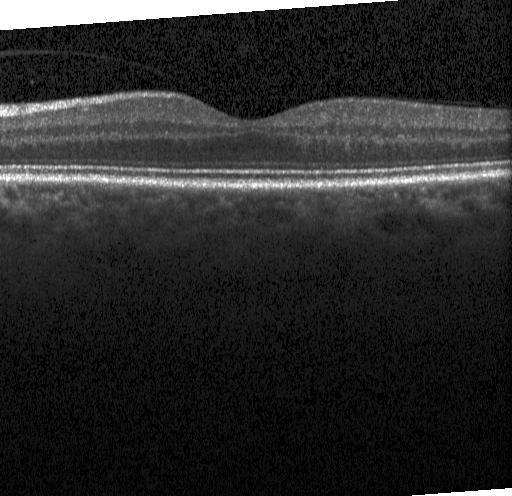
Assessment: no evidence of CNV, DME, or drusen.